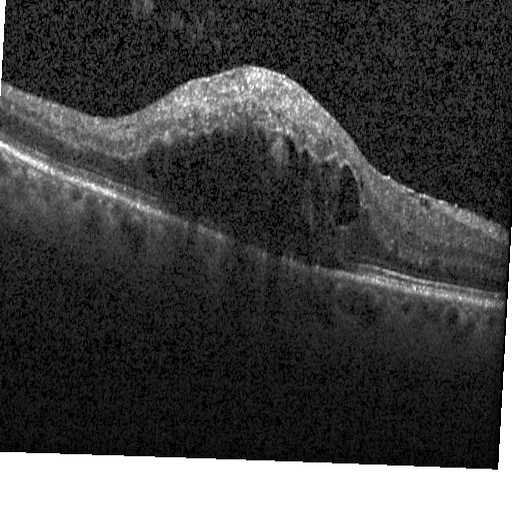

Horizontal scan through the fovea. SD-OCT. Retinal OCT cross-section. Acquired on a Heidelberg Spectralis — OCT finding: diabetic macular edema (DME).